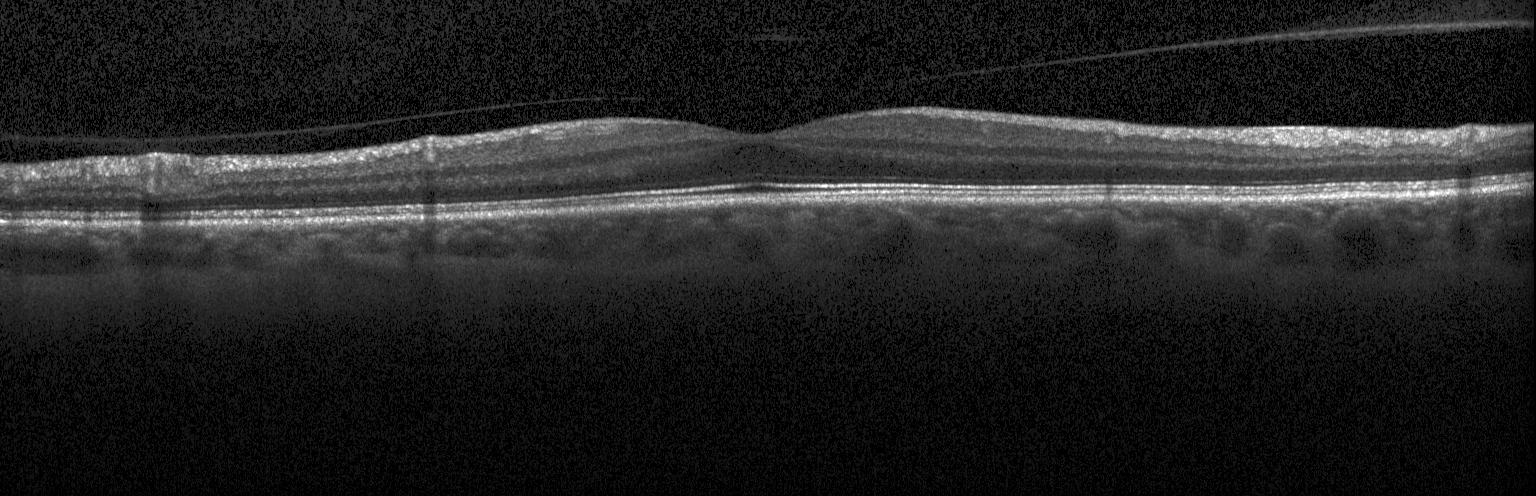
OCT finding: no choroidal neovascularization, no diabetic macular edema, and no drusen.